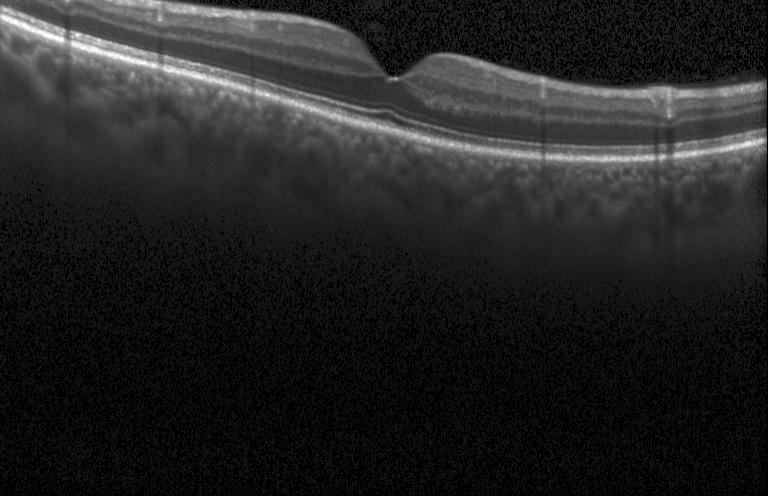 Heidelberg Spectralis; through the macula; optical coherence tomography B-scan; spectral-domain OCT. Assessment: no choroidal neovascularization, diabetic macular edema, or drusen.